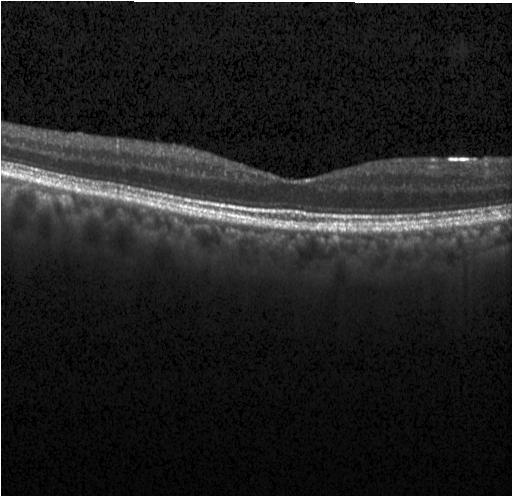

No evidence of choroidal neovascularization, diabetic macular edema, or drusen.